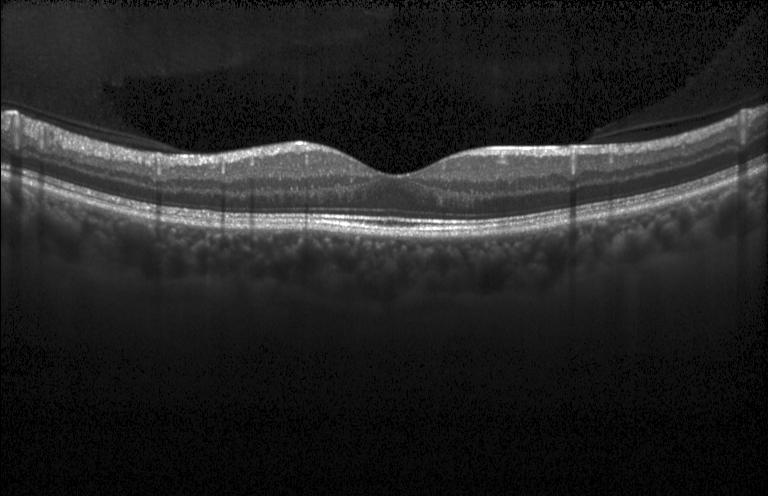

Dx: no choroidal neovascularization, diabetic macular edema, or drusen.